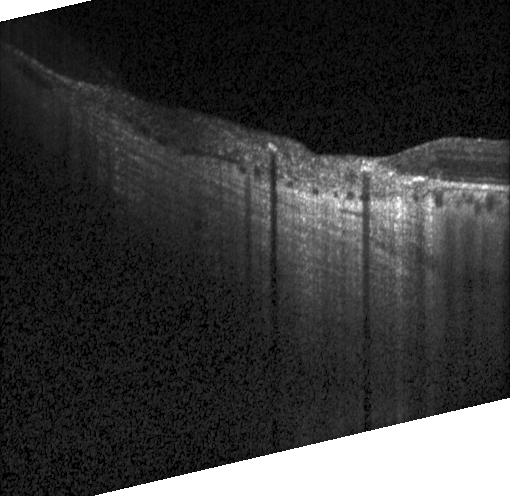 Acquired on a Heidelberg Spectralis; horizontal scan through the fovea; SD-OCT; OCT B-scan.
The scan shows choroidal neovascularization.